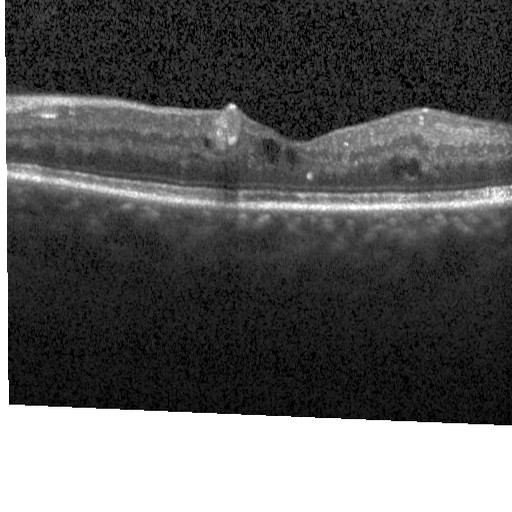 Optical coherence tomography B-scan · through the macula · acquired on a Heidelberg Spectralis. The scan shows DME.